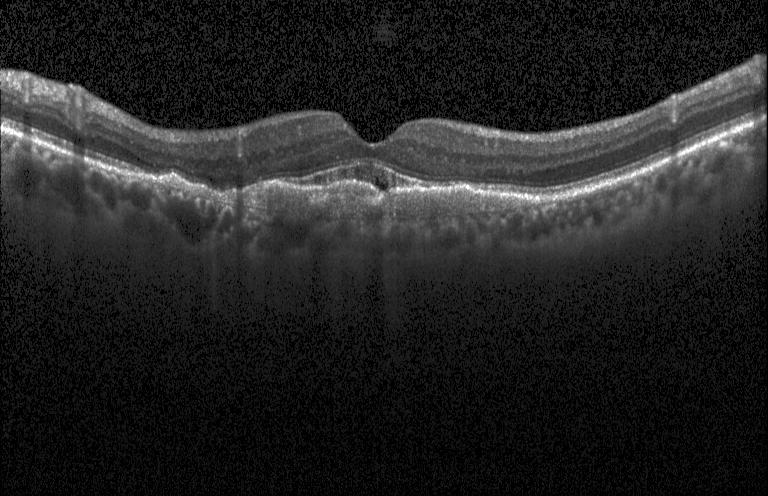
OCT line scan, spectral-domain optical coherence tomography. Finding: a choroidal neovascular membrane.